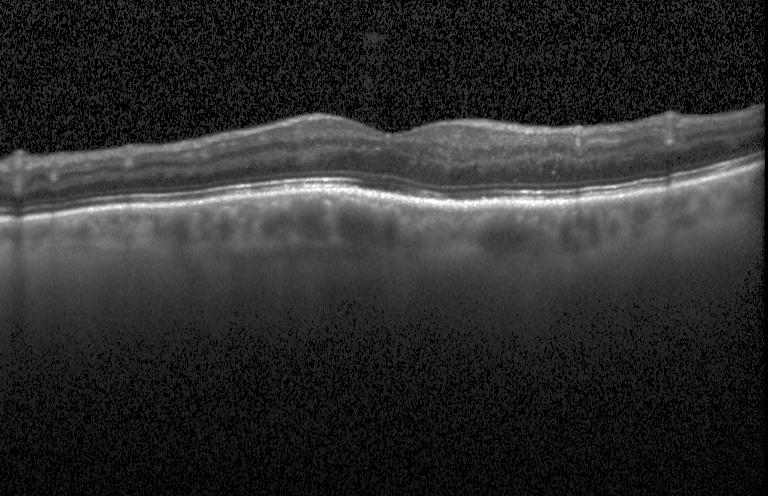

Retinal OCT cross-section — Finding: neither choroidal neovascularization, diabetic macular edema, nor drusen.